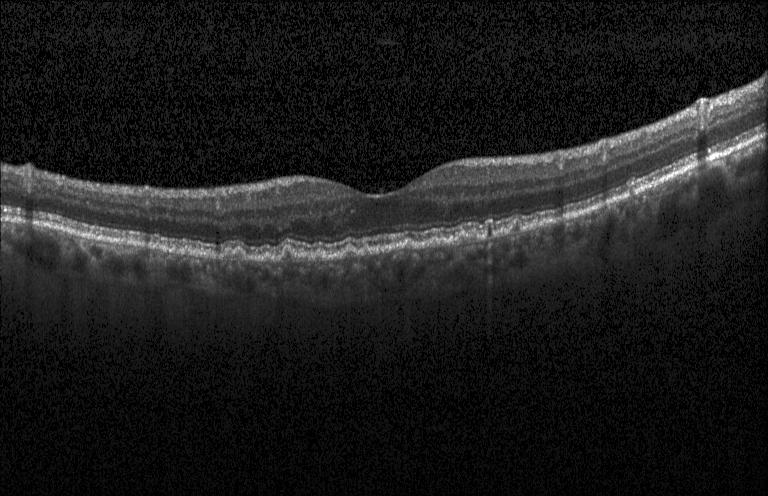 OCT line scan · Heidelberg Spectralis. Dx: sub-RPE drusenoid deposits.